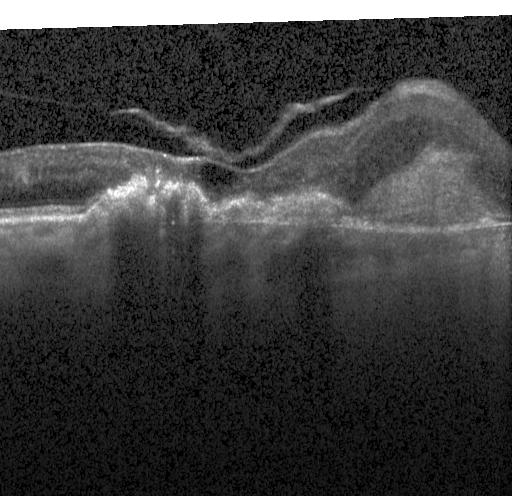
Diagnosis: CNV.